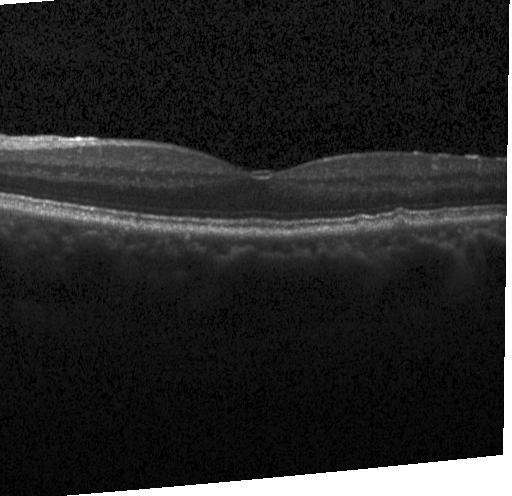
Sub-RPE drusenoid deposits.